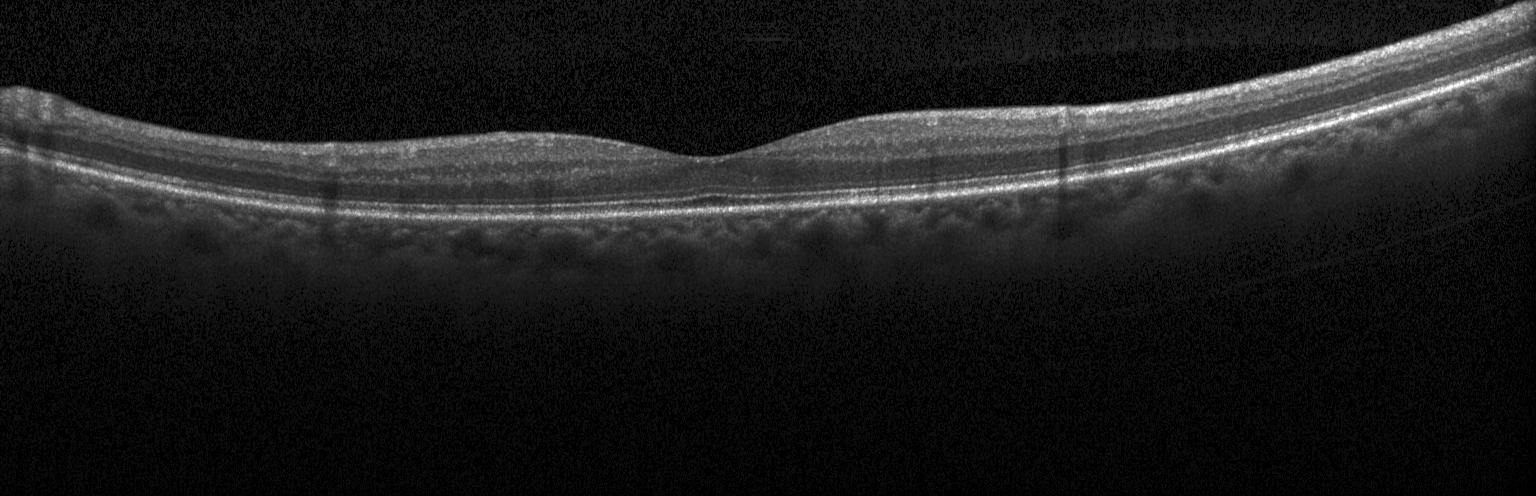 Macular scan. Heidelberg Spectralis. SD-OCT. Retinal OCT B-scan
Finding: no choroidal neovascularization, diabetic macular edema, or drusen.